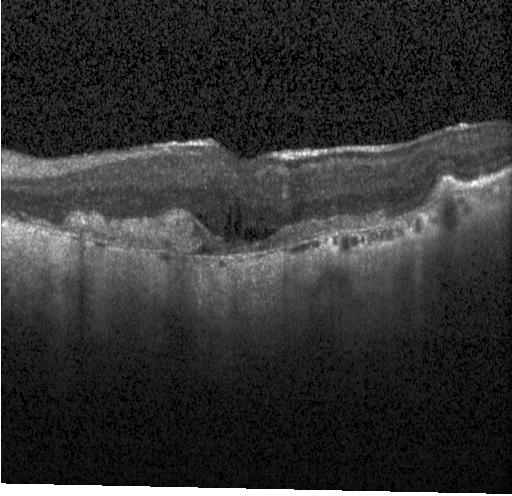 Spectral-domain OCT. Retinal OCT B-scan. Acquired on a Heidelberg Spectralis.
Choroidal neovascularization.